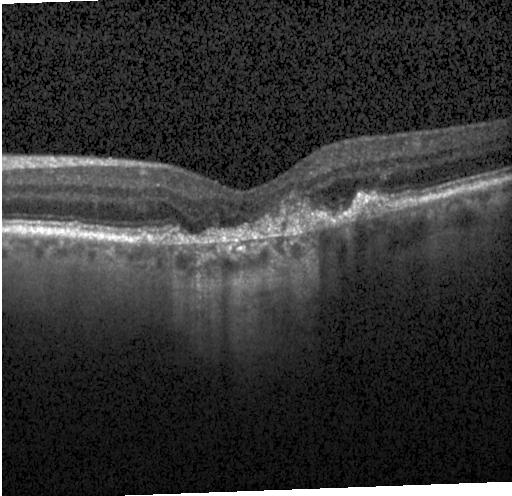
Fovea-centered. Spectral-domain OCT. Optical coherence tomography B-scan. Acquired on a Heidelberg Spectralis
This B-scan demonstrates a choroidal neovascular membrane.